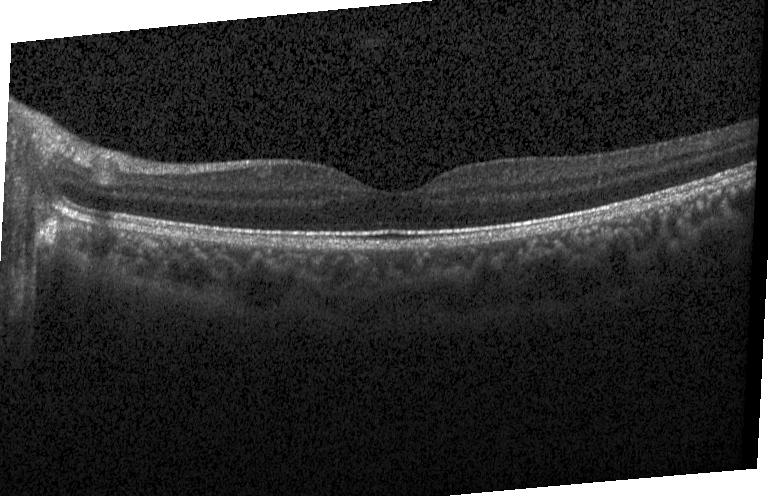
OCT line scan, Heidelberg Spectralis OCT system, through the macula, SD-OCT
No choroidal neovascularization, no diabetic macular edema, and no drusen.